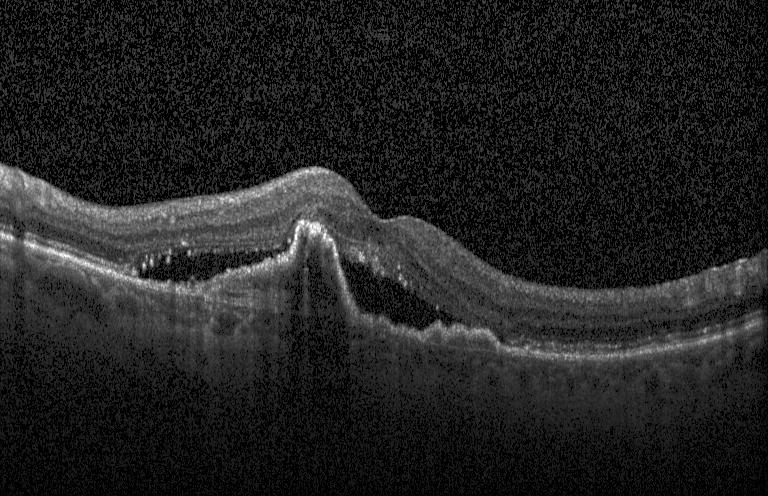
Macular OCT: choroidal neovascularization (CNV).